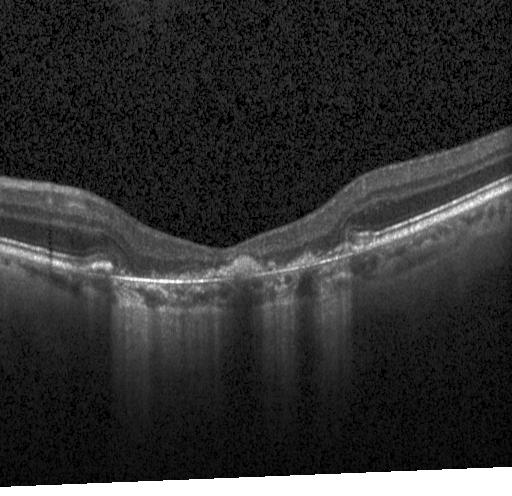 Spectral-domain optical coherence tomography. Optical coherence tomography B-scan. Horizontal scan through the fovea
Macular OCT: a choroidal neovascular membrane.